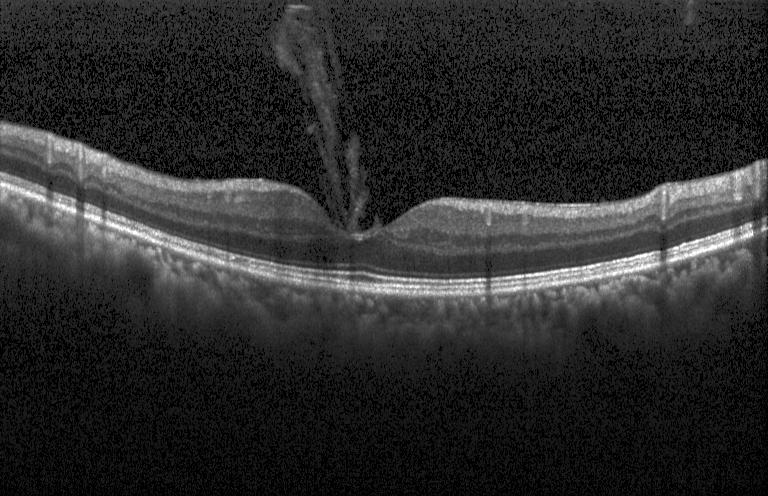

OCT scan showing no choroidal neovascularization, diabetic macular edema, or drusen.